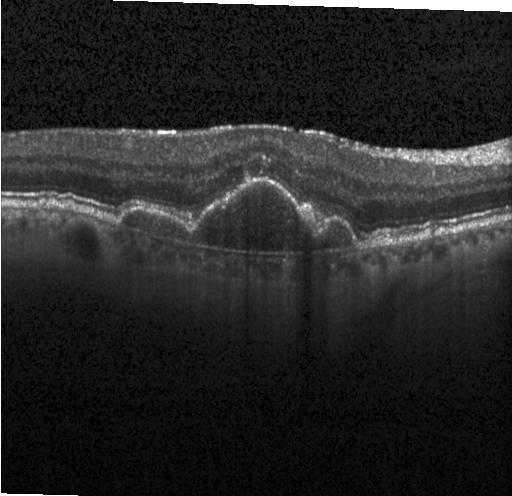

Retinal OCT B-scan
Finding: a choroidal neovascular membrane.